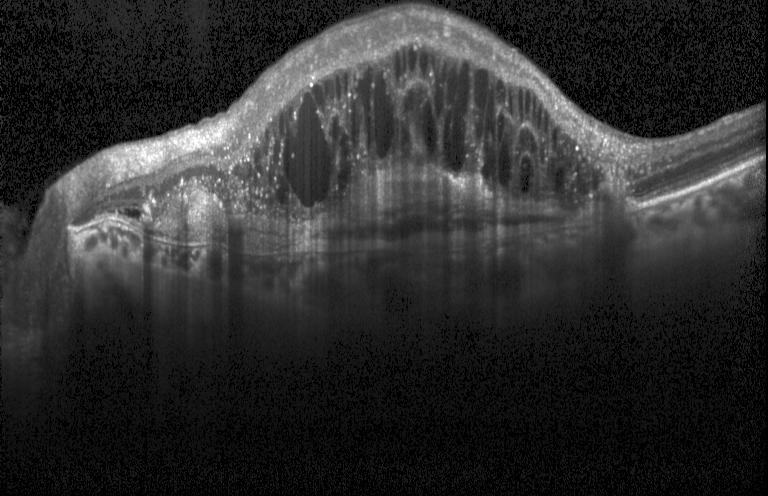
Finding: DME.